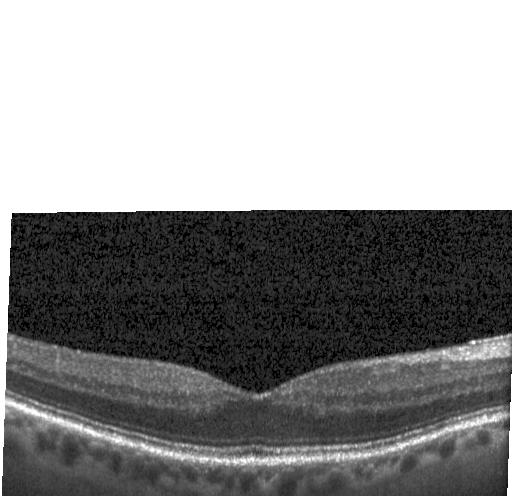

OCT B-scan — Diagnosis: no choroidal neovascularization, diabetic macular edema, or drusen.